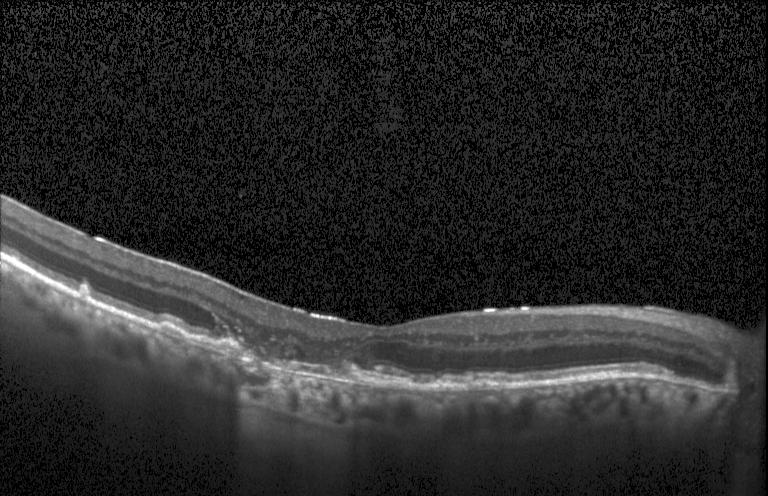

Retinal OCT cross-section; acquired on a Heidelberg Spectralis — Impression: choroidal neovascularization.